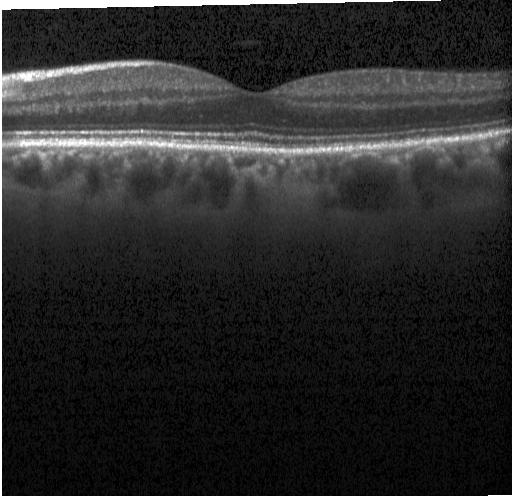

Dx: no choroidal neovascularization, no diabetic macular edema, and no drusen.